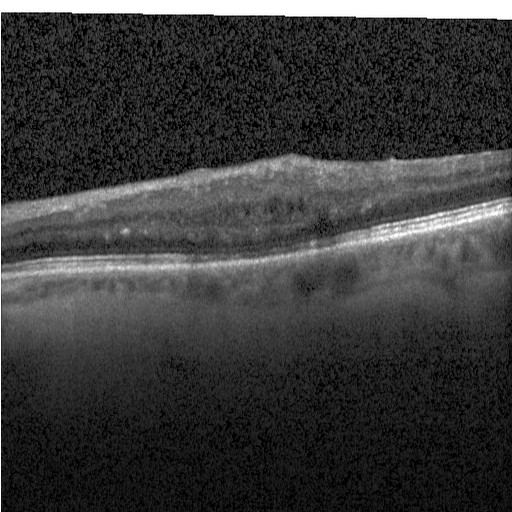 OCT scan showing DME.